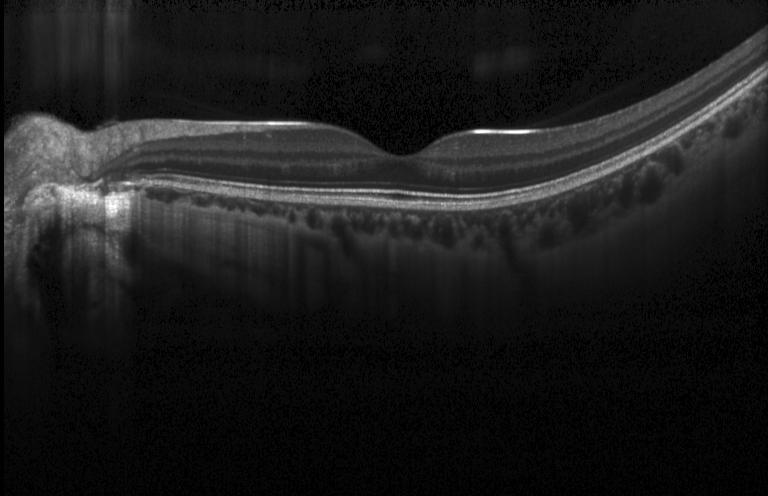
Macular OCT demonstrating no CNV, no DME, and no drusen.